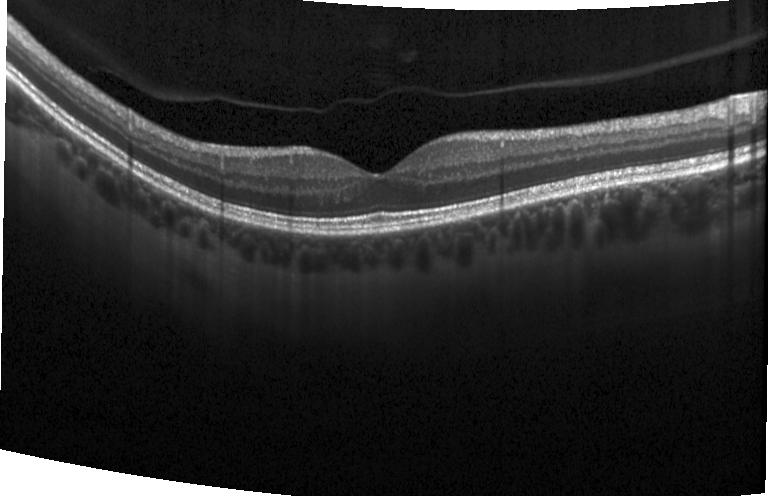

Retinal OCT B-scan. SD-OCT. Fovea-centered
OCT finding: no choroidal neovascularization, diabetic macular edema, or drusen.